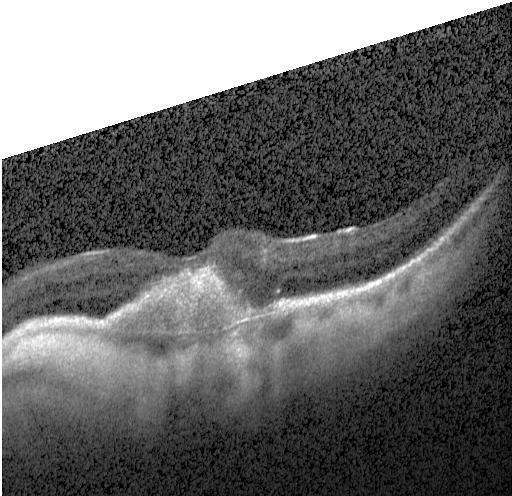
OCT line scan, instrument: Heidelberg Spectralis — OCT finding: choroidal neovascularization (CNV).